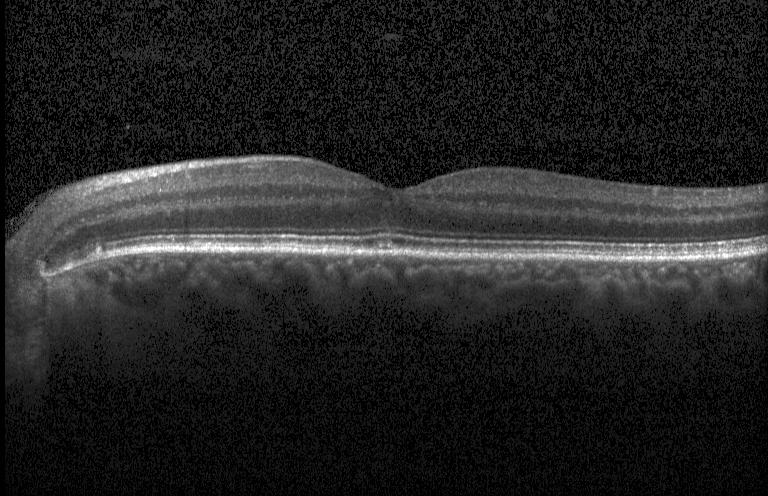
Retinal OCT cross-section showing neither choroidal neovascularization, diabetic macular edema, nor drusen.